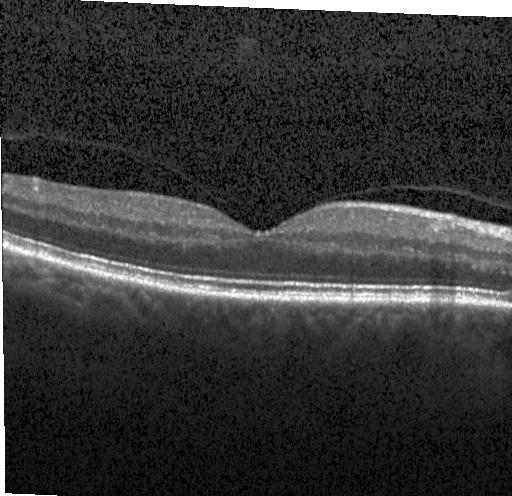

Optical coherence tomography scan. Spectral-domain optical coherence tomography.
Dx: no CNV, DME, or drusen.